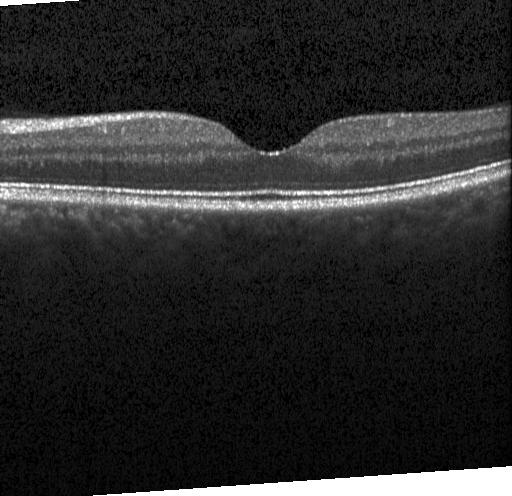

Heidelberg Spectralis OCT system · retinal OCT B-scan. Macular OCT: no CNV, no DME, and no drusen.